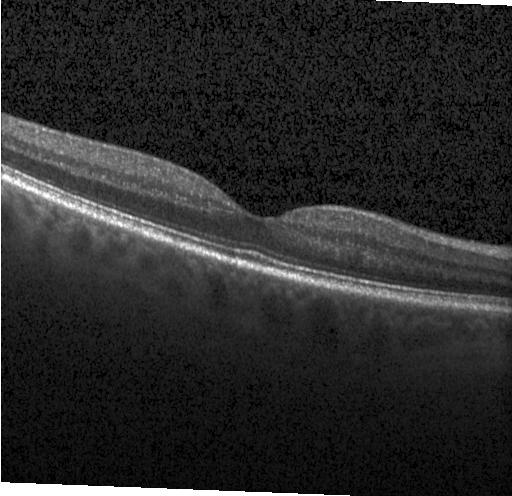

OCT B-scan showing no evidence of choroidal neovascularization, diabetic macular edema, or drusen.